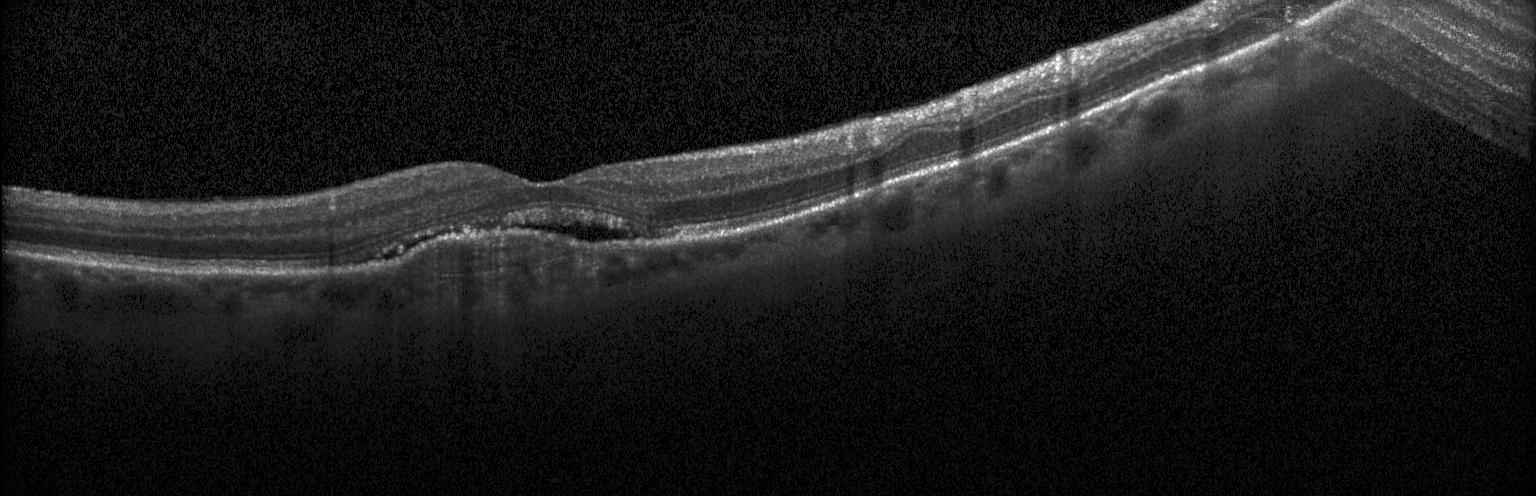 Optical coherence tomography scan; Heidelberg Spectralis; spectral-domain OCT. OCT finding: CNV.